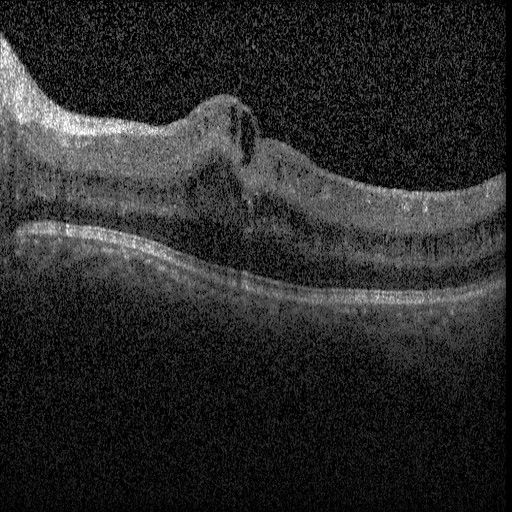 OCT B-scan — Macular OCT: diabetic macular edema (DME).